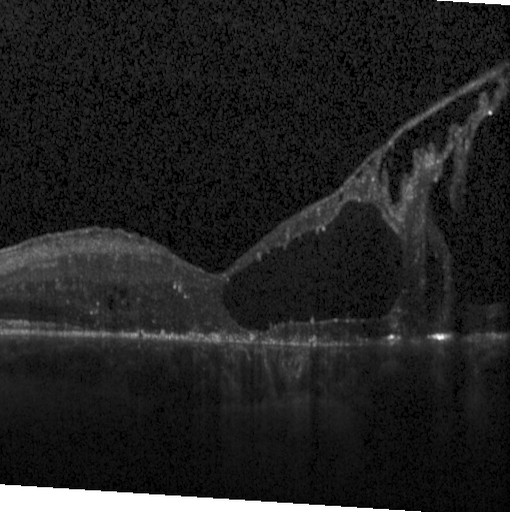

Retinal OCT cross-section · horizontal scan through the fovea · SD-OCT · Heidelberg Spectralis OCT system
Macular OCT: diabetic macular edema (DME).